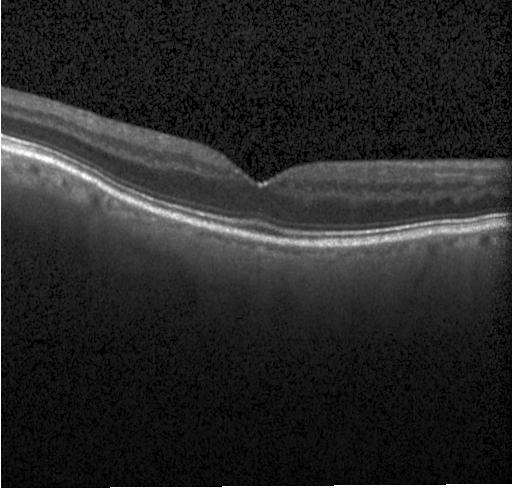

The scan shows no CNV, no DME, and no drusen.